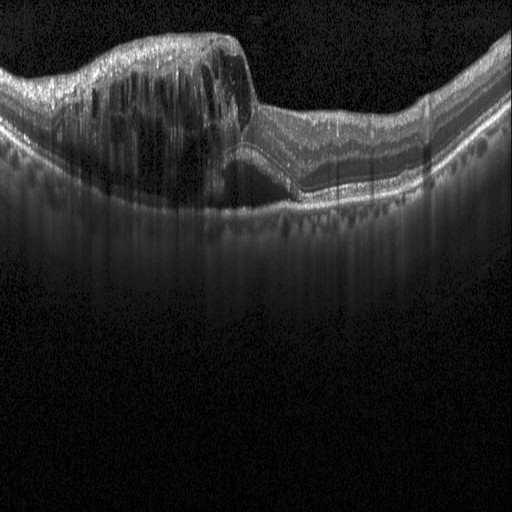

Through the macula, OCT line scan, Heidelberg Spectralis OCT system.
Impression: diabetic macular edema.